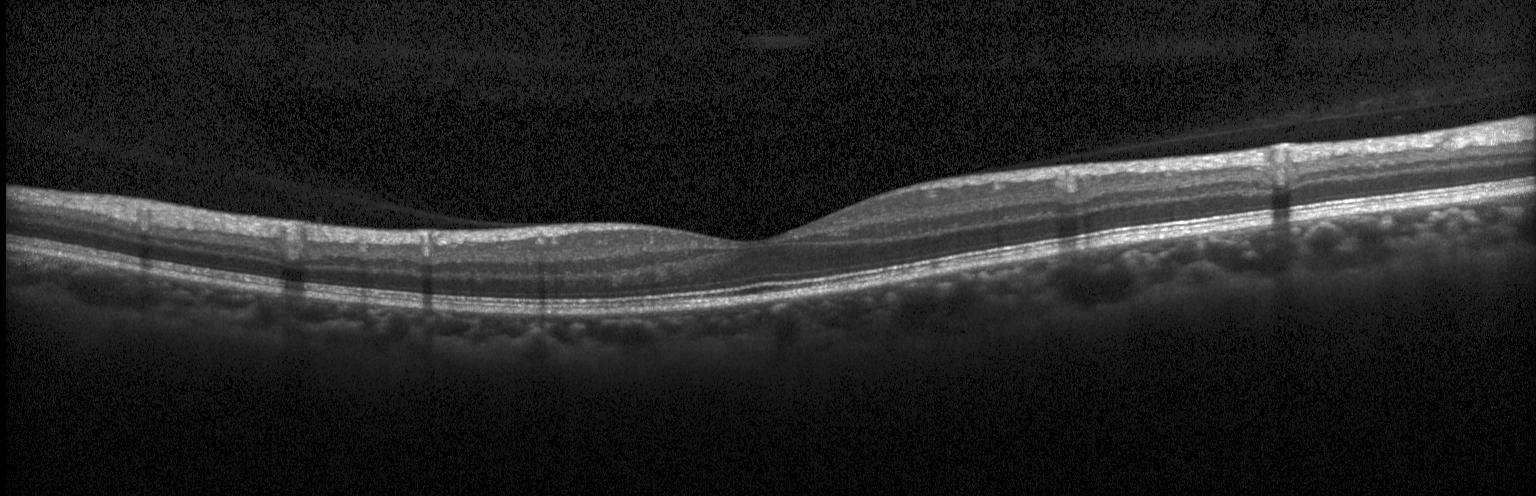

Optical coherence tomography B-scan; spectral-domain optical coherence tomography; fovea-centered; Heidelberg Spectralis OCT system.
OCT finding: no CNV, DME, or drusen.